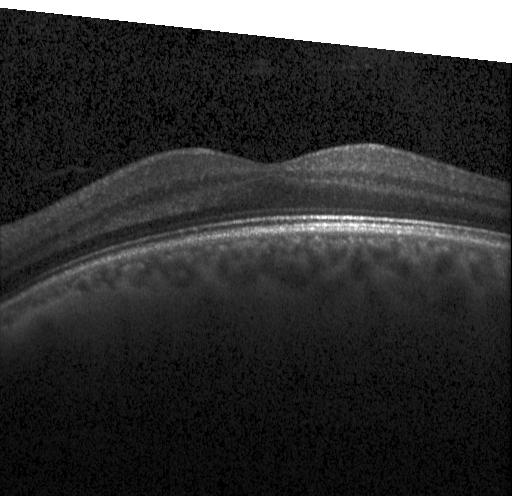 Optical coherence tomography scan · spectral-domain OCT · macular scan — OCT finding: no choroidal neovascularization, no diabetic macular edema, and no drusen.